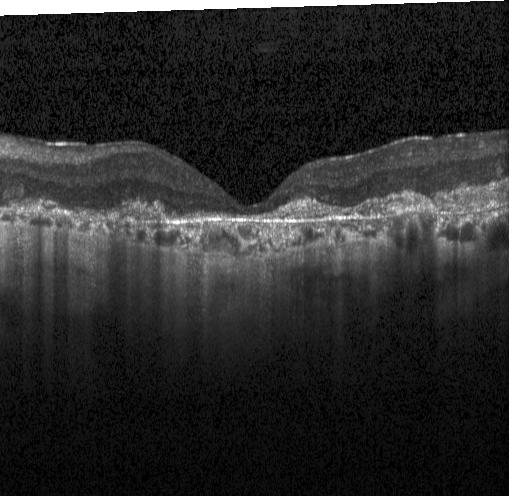 Acquired on a Heidelberg Spectralis; SD-OCT; centered on the fovea; optical coherence tomography B-scan.
Impression: a choroidal neovascular membrane.